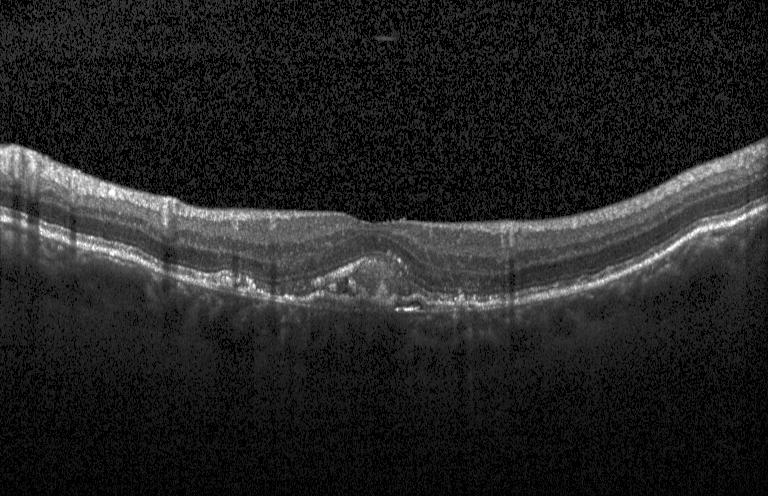

Impression: CNV.